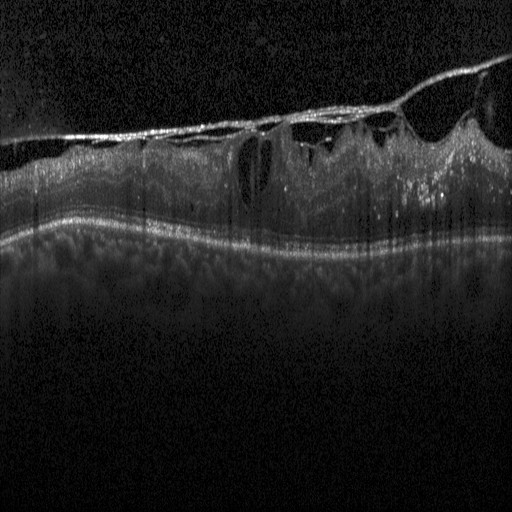

Assessment: diabetic macular edema (DME).